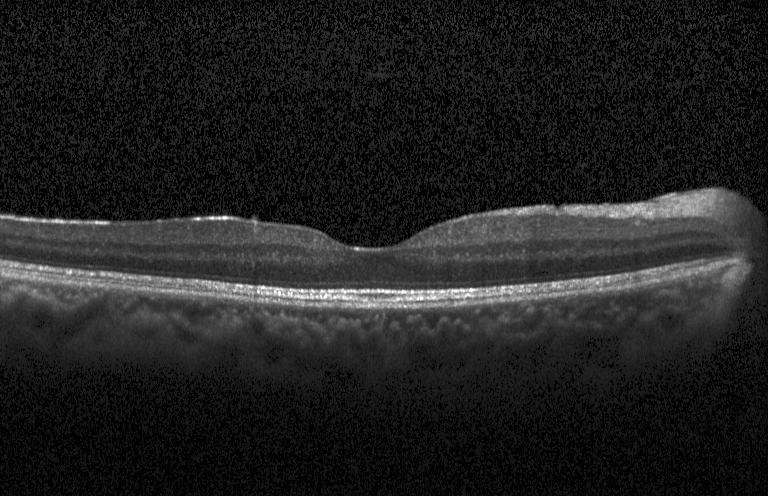 Optical coherence tomography scan. Diagnosis: no evidence of CNV, DME, or drusen.